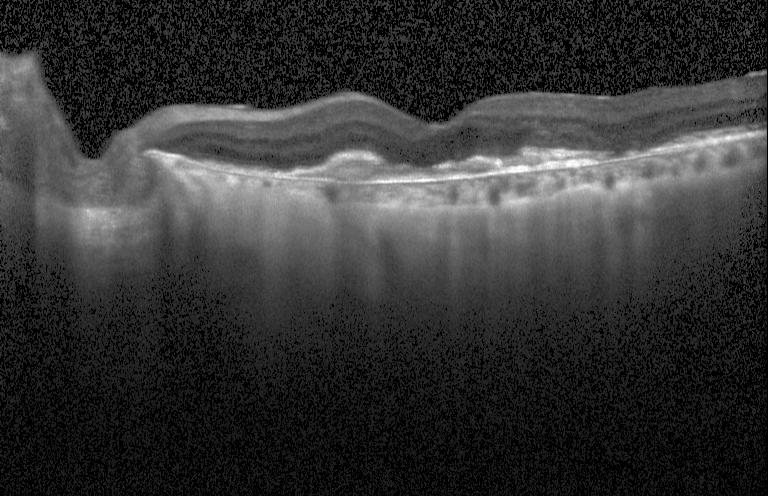

Diagnosis: CNV.